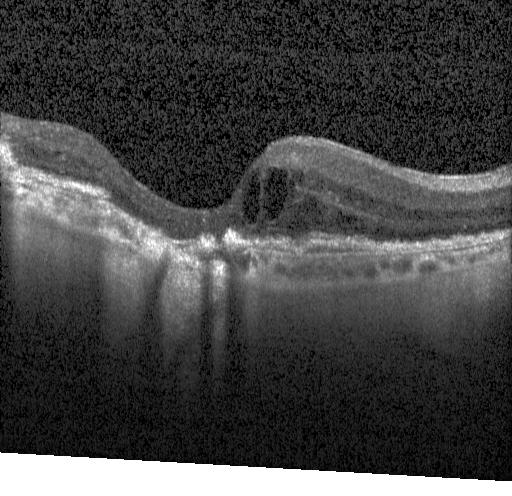
A choroidal neovascular membrane.